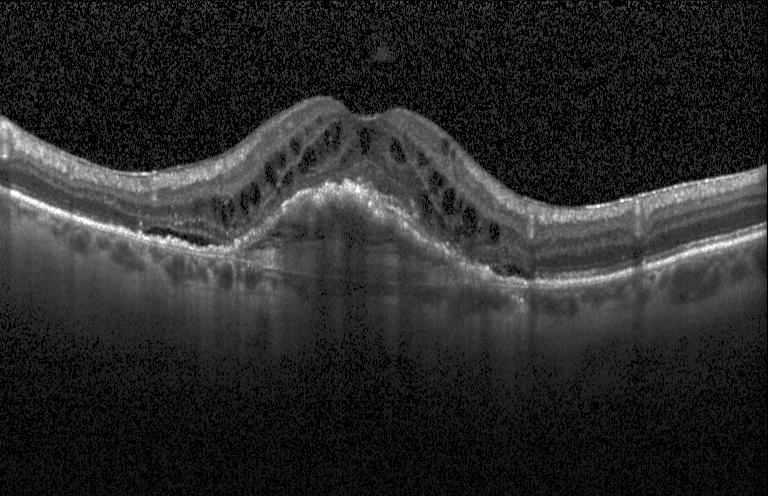
Spectral-domain optical coherence tomography. Through the macula. Heidelberg Spectralis OCT system. Optical coherence tomography scan.
Assessment: a choroidal neovascular membrane.